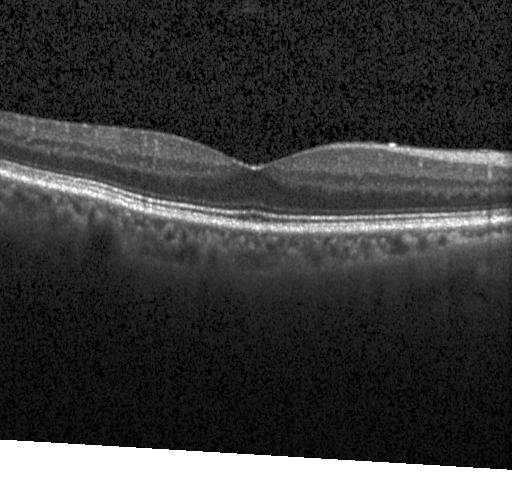
Optical coherence tomography scan
Dx: no choroidal neovascularization, diabetic macular edema, or drusen.